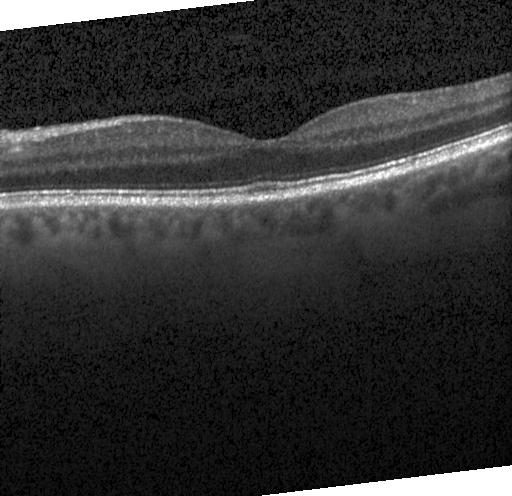
Instrument: Heidelberg Spectralis. SD-OCT. OCT B-scan
Diagnosis: neither choroidal neovascularization, diabetic macular edema, nor drusen.